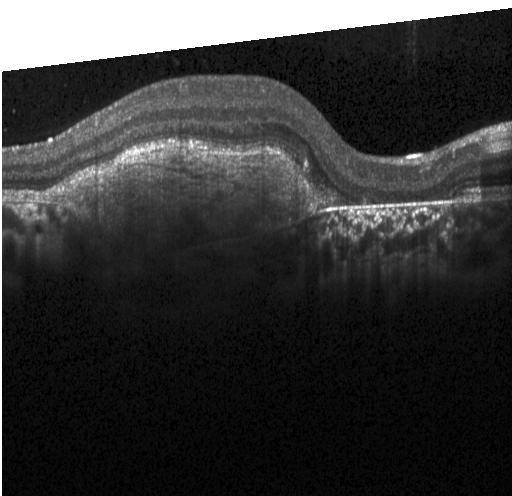

Spectral-domain OCT B-scan: choroidal neovascularization (CNV).